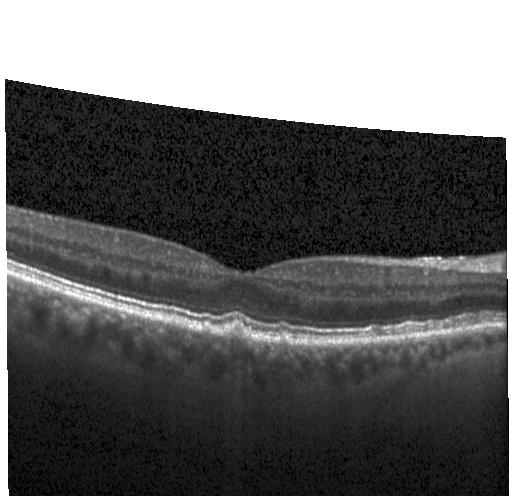
Optical coherence tomography B-scan. Diagnosis: multiple drusen.